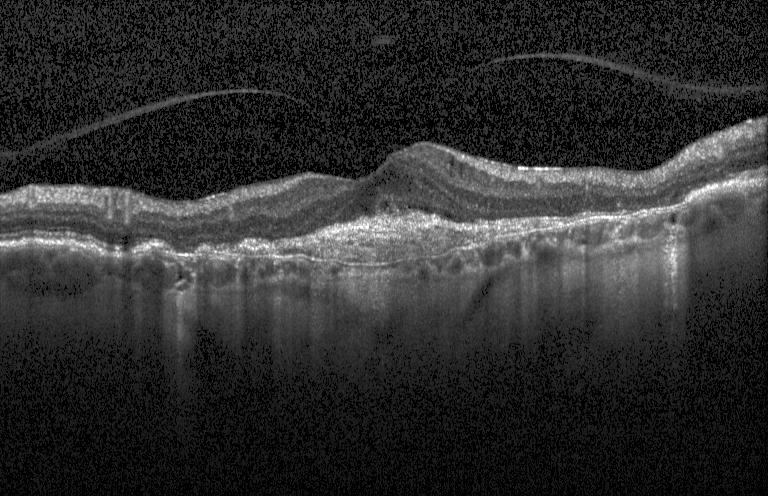
Diagnosis: choroidal neovascularization (CNV).